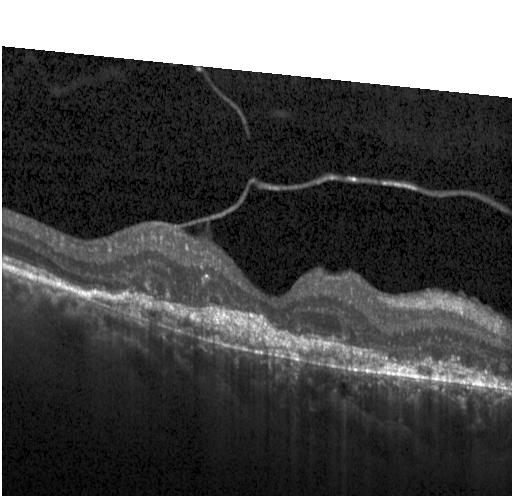

Finding: a choroidal neovascular membrane.